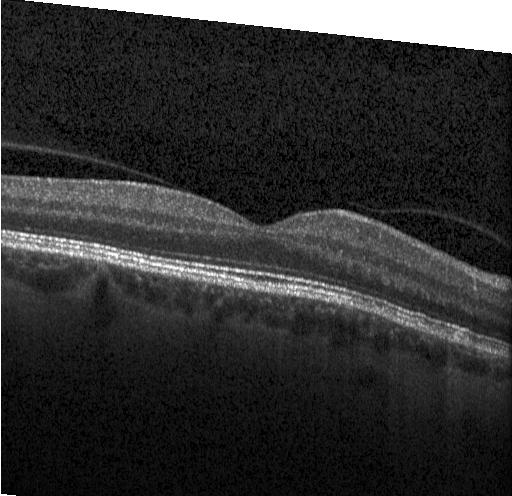 Horizontal scan through the fovea; OCT B-scan; acquired on a Heidelberg Spectralis; SD-OCT
Neither choroidal neovascularization, diabetic macular edema, nor drusen.